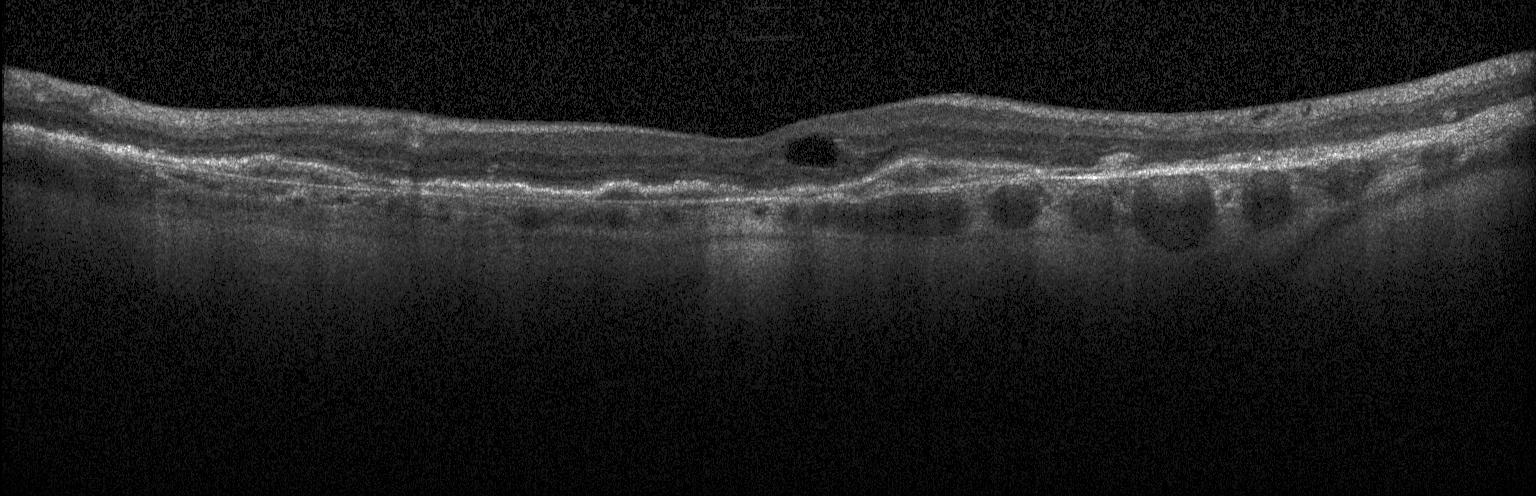

Macular scan, retinal OCT cross-section. Diagnosis: a choroidal neovascular membrane.